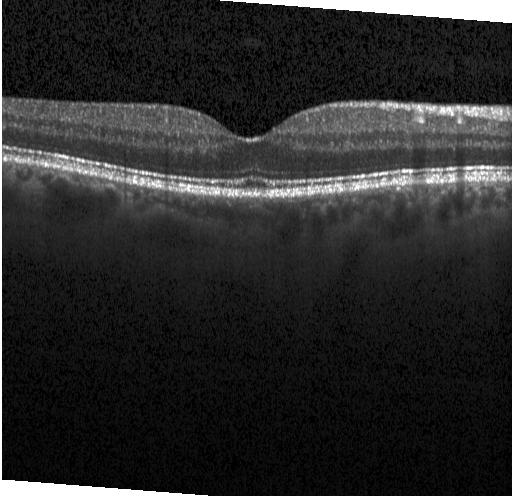

Optical coherence tomography B-scan.
Diagnosis: neither choroidal neovascularization, diabetic macular edema, nor drusen.